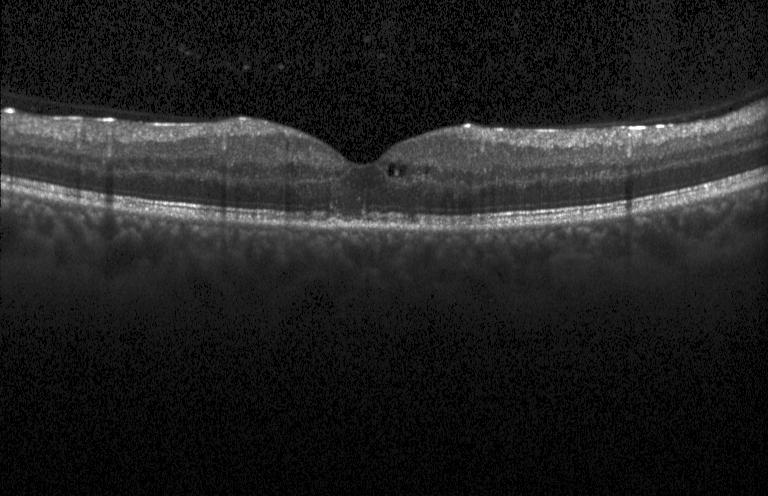 OCT line scan — Macular OCT: diabetic macular edema.